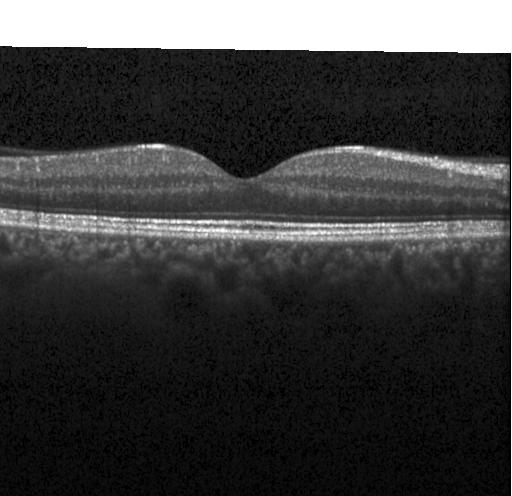
Retinal OCT cross-section; spectral-domain OCT; acquired on a Heidelberg Spectralis. Dx: no CNV, DME, or drusen.